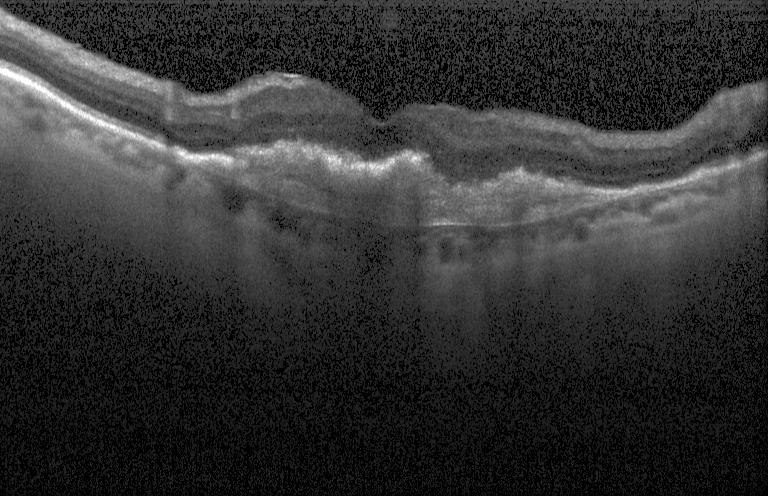

Heidelberg Spectralis · centered on the fovea · OCT B-scan — The scan shows CNV.